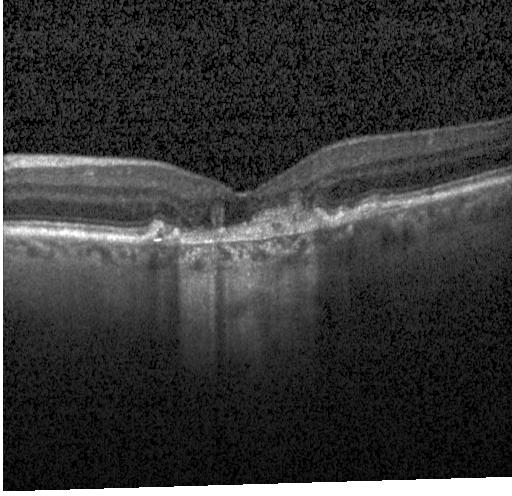

Dx: choroidal neovascularization (CNV).